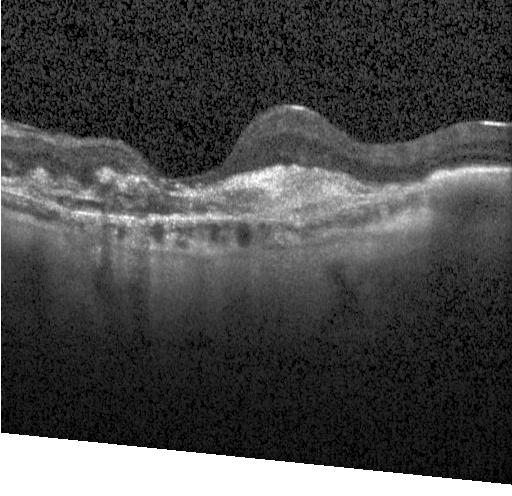

OCT B-scan showing a choroidal neovascular membrane.